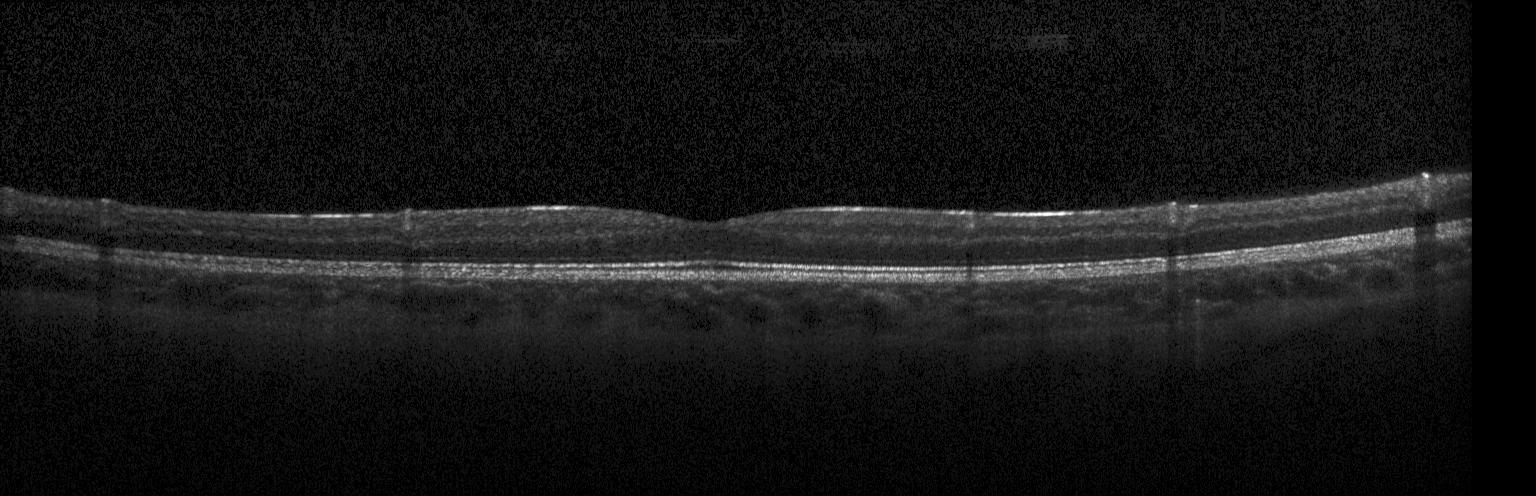

Instrument: Heidelberg Spectralis, spectral-domain OCT, retinal OCT B-scan, horizontal scan through the fovea
Diagnosis: neither CNV, DME, nor drusen.